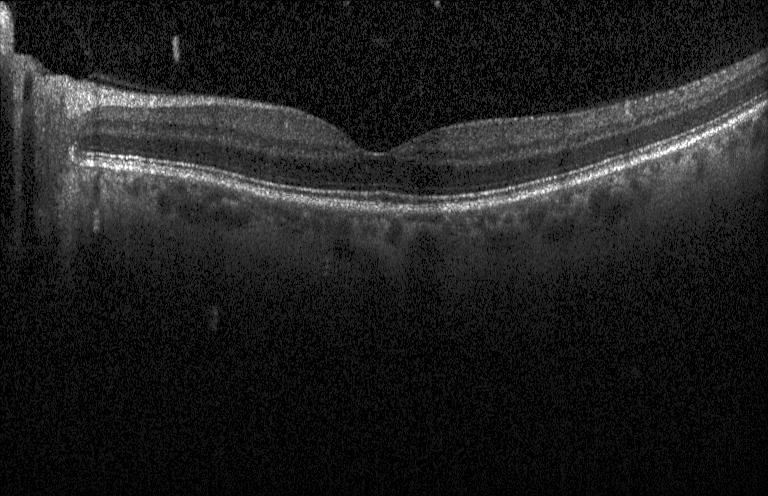

Heidelberg Spectralis OCT system; centered on the fovea; optical coherence tomography B-scan.
No choroidal neovascularization, diabetic macular edema, or drusen.